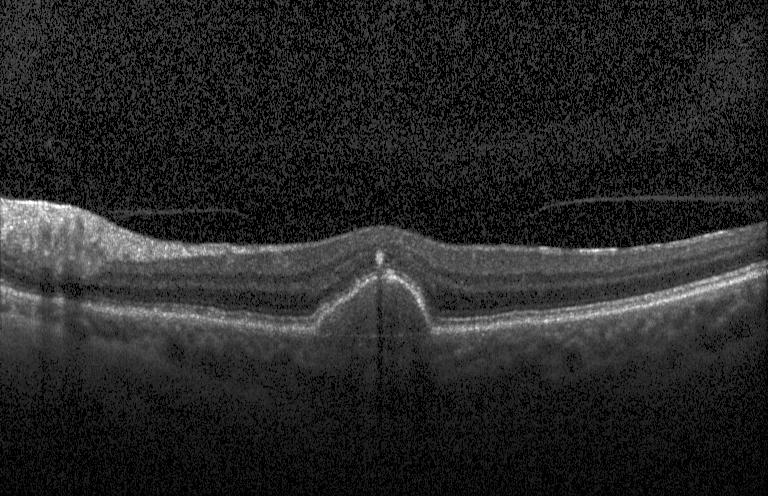

OCT B-scan. This B-scan demonstrates CNV.